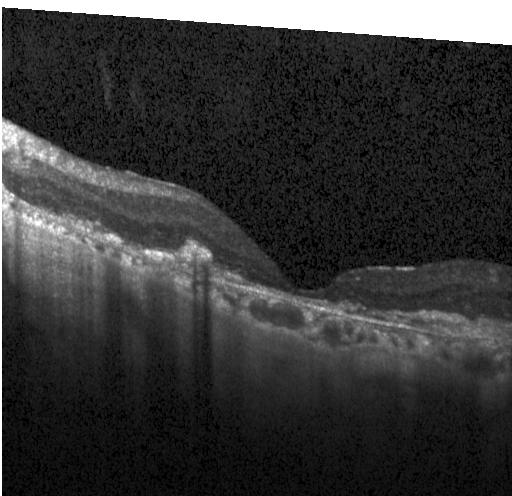
Centered on the fovea · OCT line scan · spectral-domain OCT · Heidelberg Spectralis OCT system. CNV.